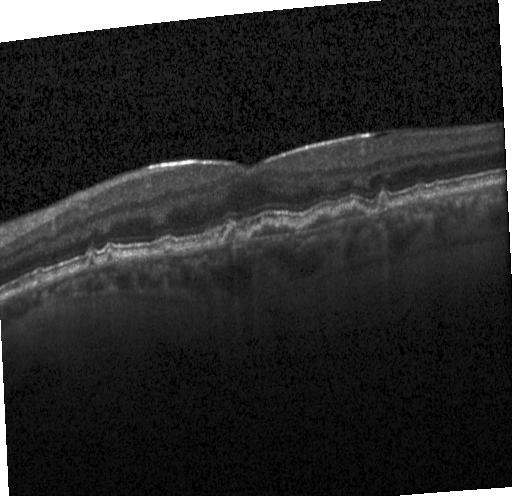 Retinal OCT B-scan — This B-scan demonstrates multiple drusen.